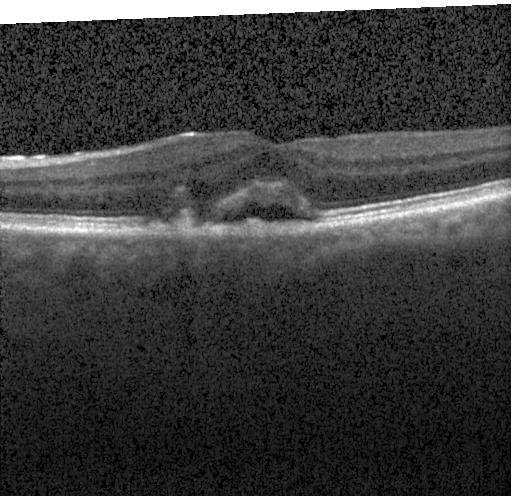
OCT line scan.
OCT finding: CNV.